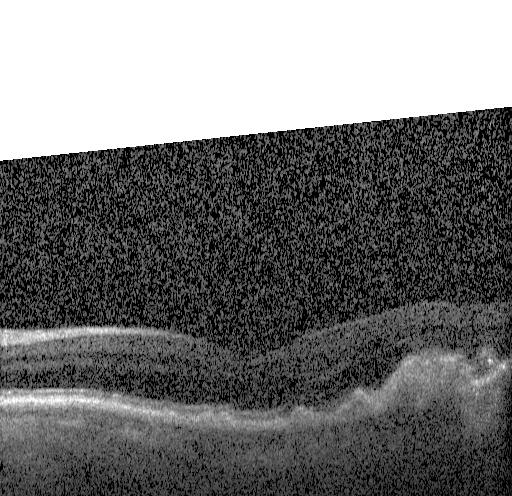
SD-OCT. Fovea-centered. OCT B-scan
Impression: a choroidal neovascular membrane.